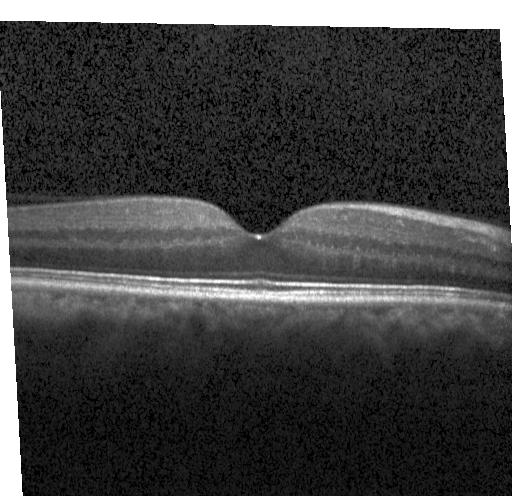 Optical coherence tomography B-scan · horizontal scan through the fovea · instrument: Heidelberg Spectralis · SD-OCT
Assessment: no evidence of choroidal neovascularization, diabetic macular edema, or drusen.